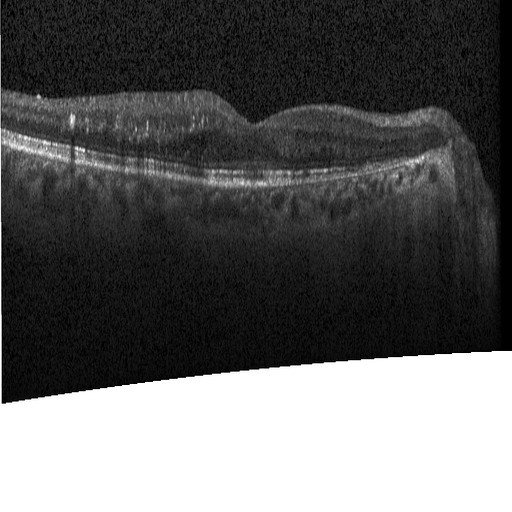

Assessment: diabetic macular edema (DME).